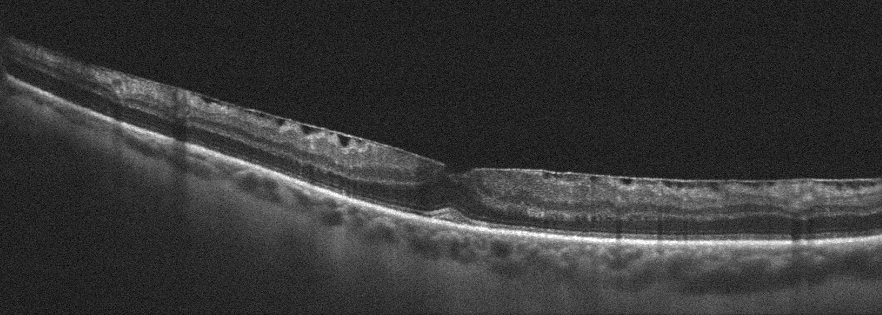 Finding: ERM.